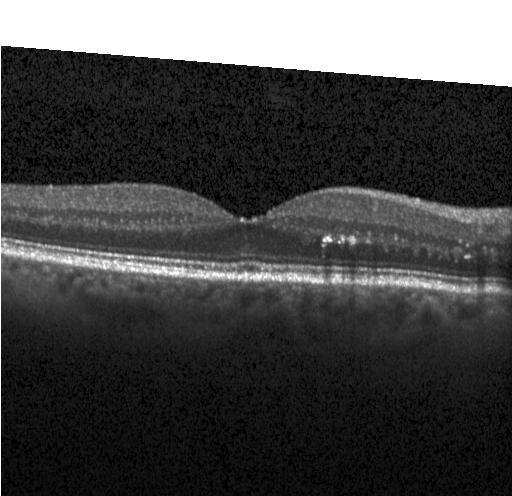
OCT line scan — The scan shows no choroidal neovascularization, no diabetic macular edema, and no drusen.